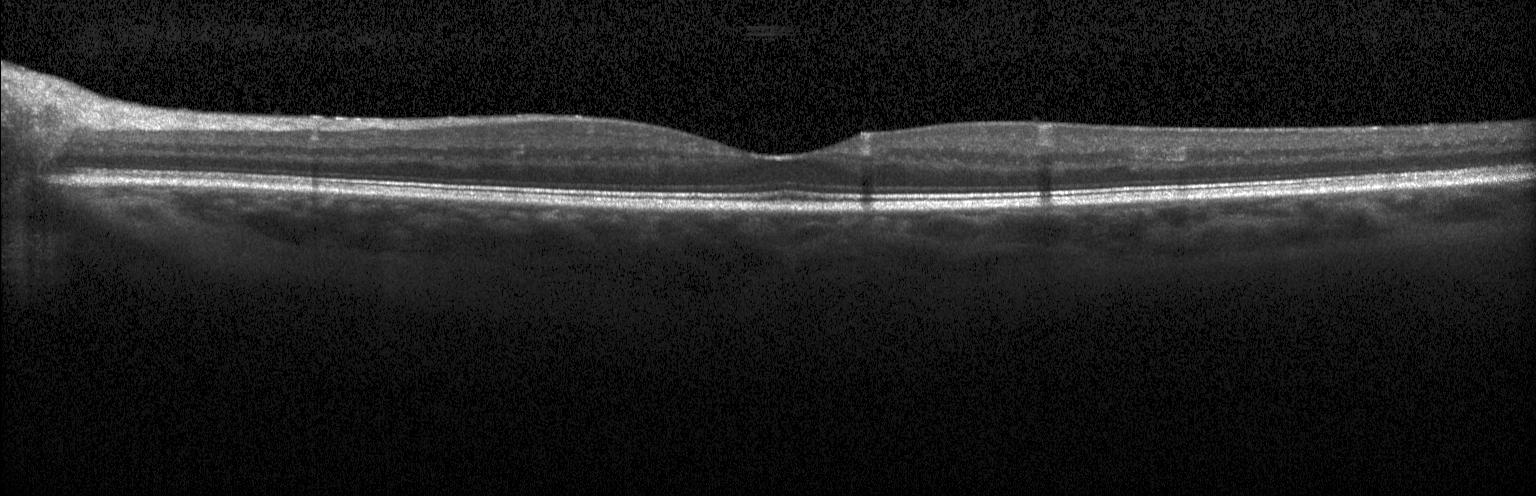 Finding: no choroidal neovascularization, no diabetic macular edema, and no drusen.